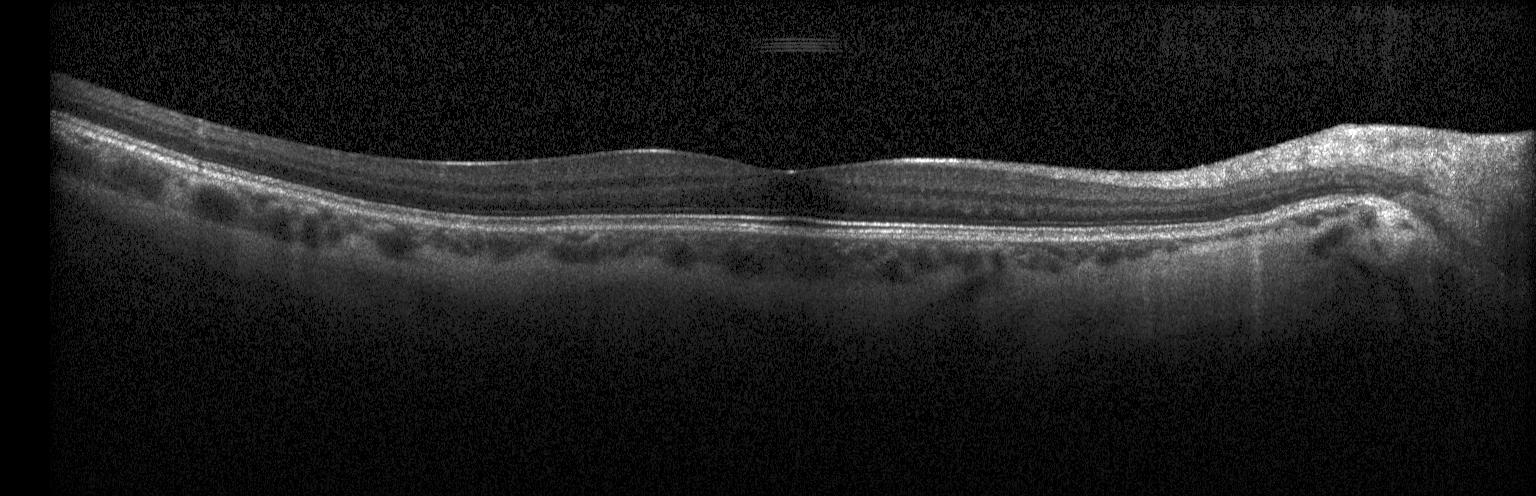
Heidelberg Spectralis, optical coherence tomography scan, fovea-centered. Impression: no choroidal neovascularization, diabetic macular edema, or drusen.